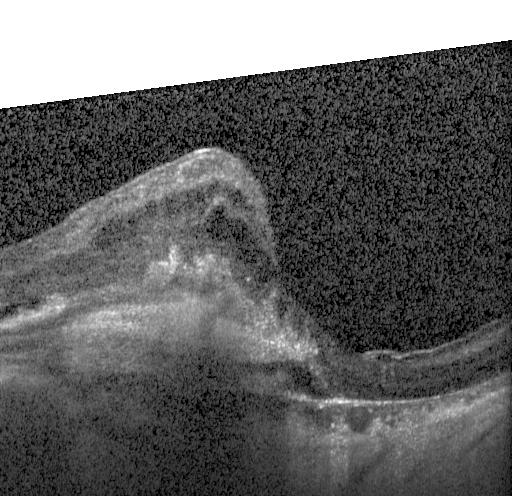 A choroidal neovascular membrane.